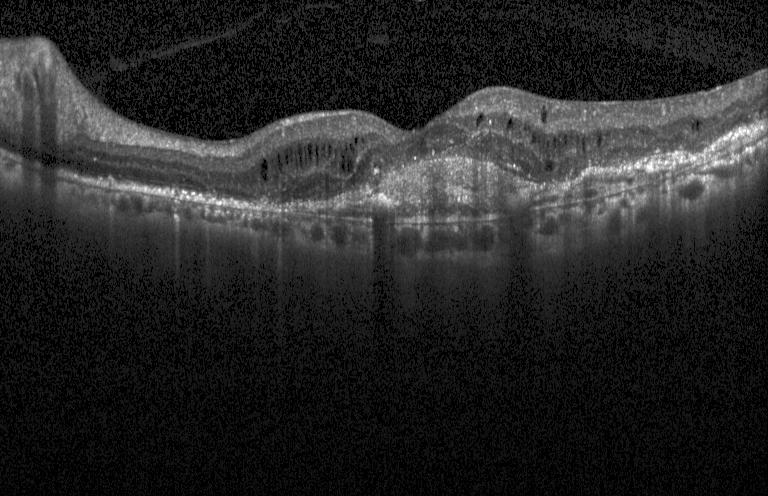 Diagnosis: a choroidal neovascular membrane.